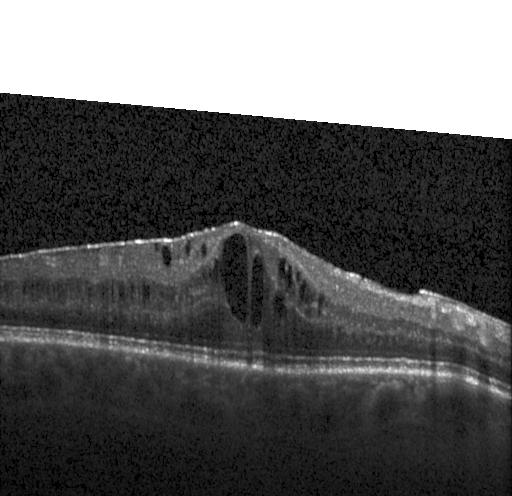 Finding: diabetic macular edema.